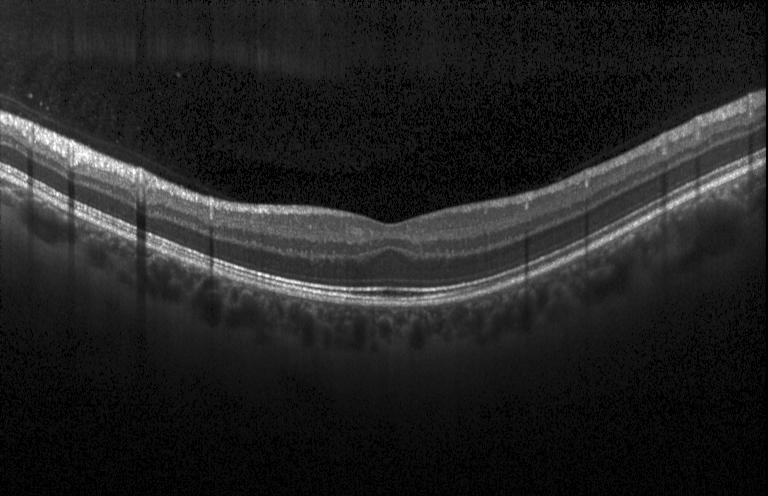 OCT line scan
Finding: no choroidal neovascularization, no diabetic macular edema, and no drusen.